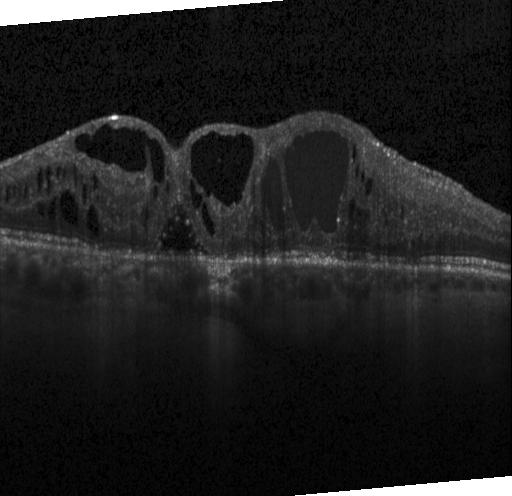
Diagnosis: diabetic macular edema.